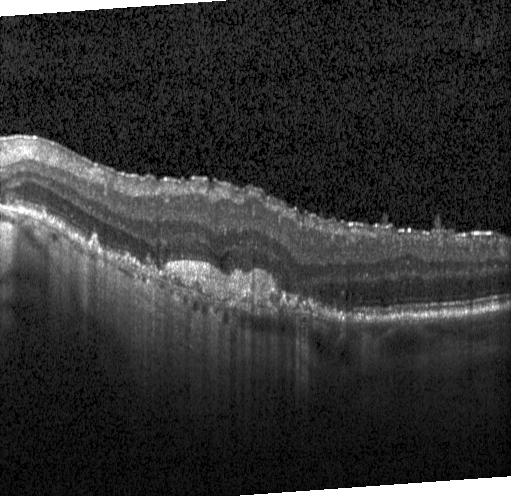
Optical coherence tomography B-scan
Impression: a choroidal neovascular membrane.